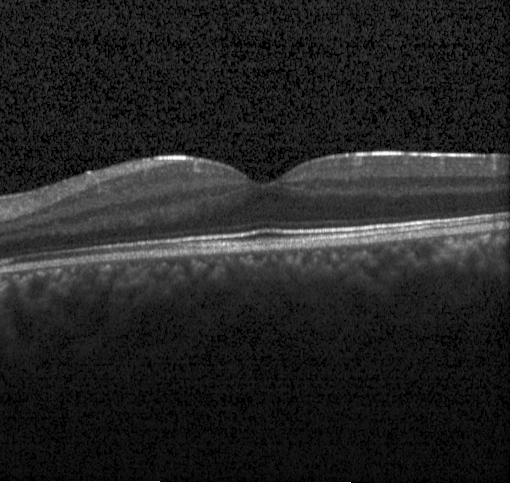 Spectral-domain optical coherence tomography, optical coherence tomography B-scan, through the macula. Dx: neither choroidal neovascularization, diabetic macular edema, nor drusen.